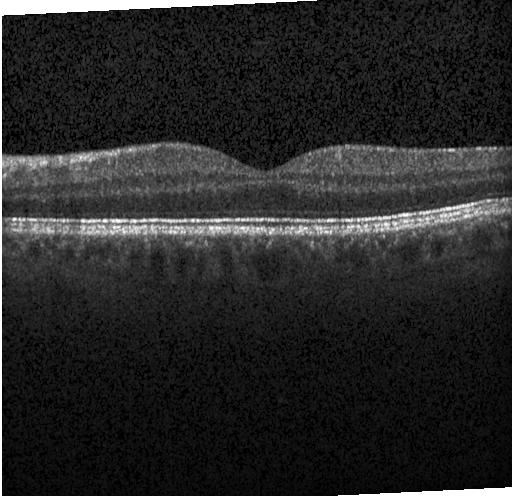
OCT B-scan, spectral-domain OCT — Diagnosis: no choroidal neovascularization, no diabetic macular edema, and no drusen.